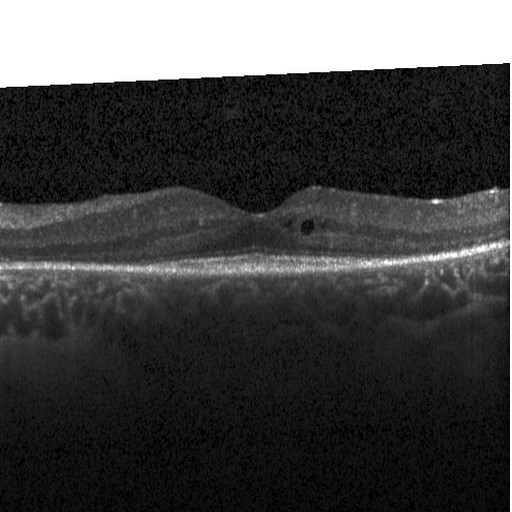

Finding: diabetic macular edema (DME).